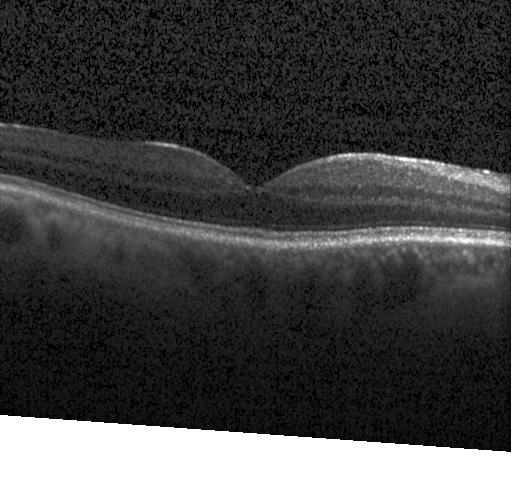

Finding: no evidence of choroidal neovascularization, diabetic macular edema, or drusen.